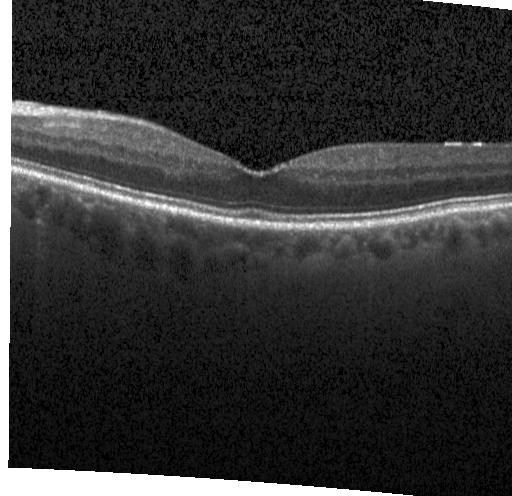
Horizontal scan through the fovea, Heidelberg Spectralis, spectral-domain optical coherence tomography, OCT line scan.
Macular OCT: no choroidal neovascularization, diabetic macular edema, or drusen.